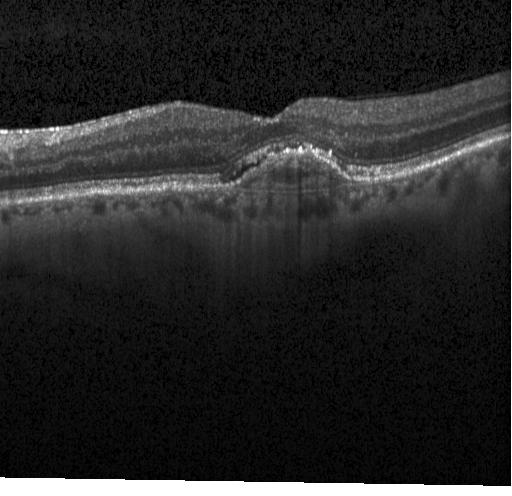

Optical coherence tomography scan.
Finding: a choroidal neovascular membrane.